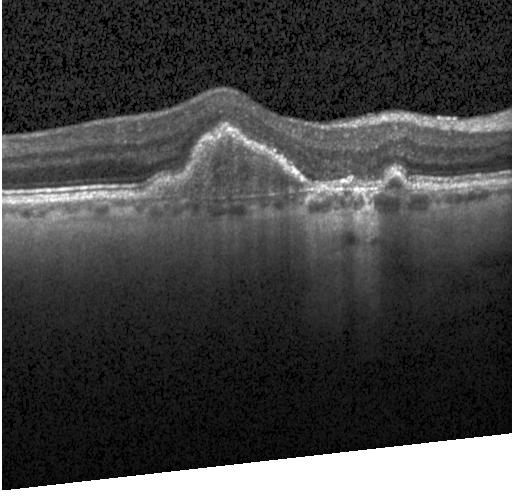

Macular OCT demonstrating a choroidal neovascular membrane.